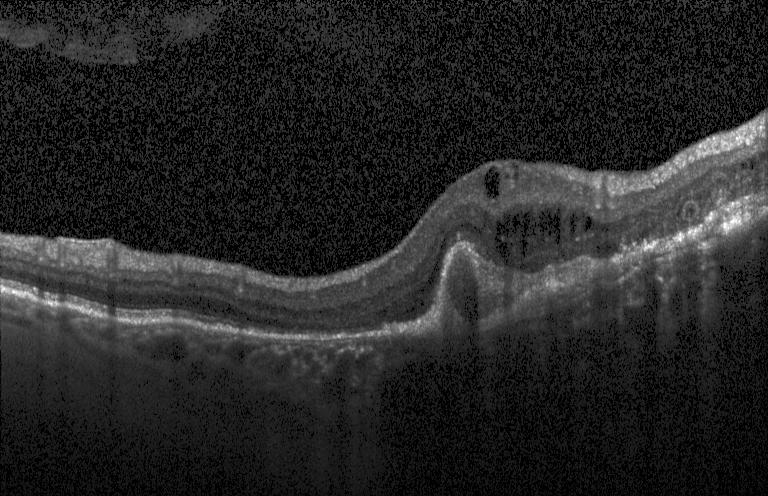
OCT B-scan · through the macula — Diagnosis: choroidal neovascularization (CNV).